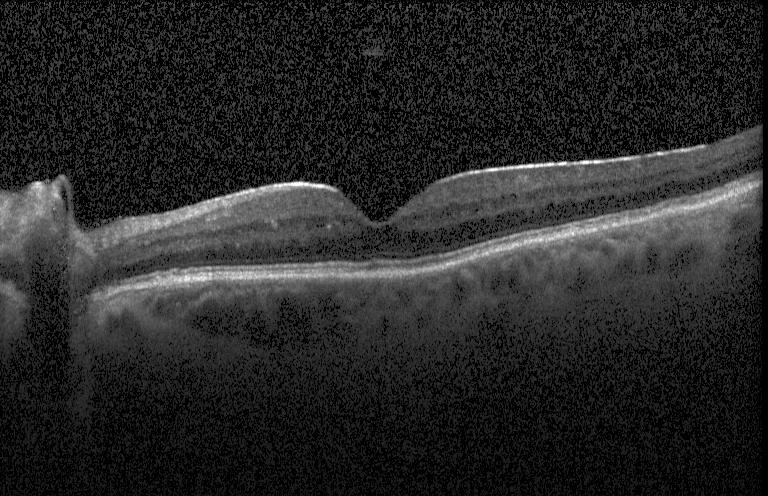
Optical coherence tomography scan
No choroidal neovascularization, diabetic macular edema, or drusen.